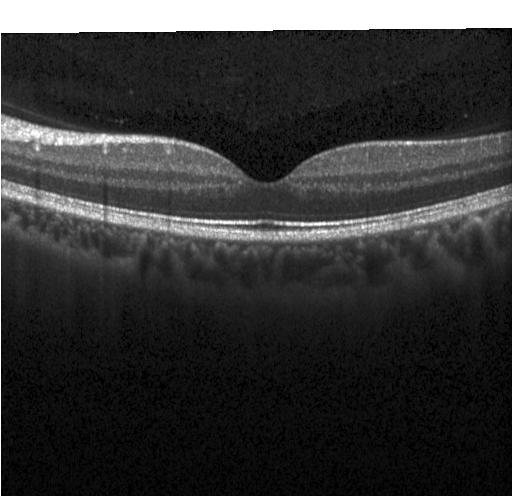 Optical coherence tomography B-scan — Finding: no CNV, DME, or drusen.